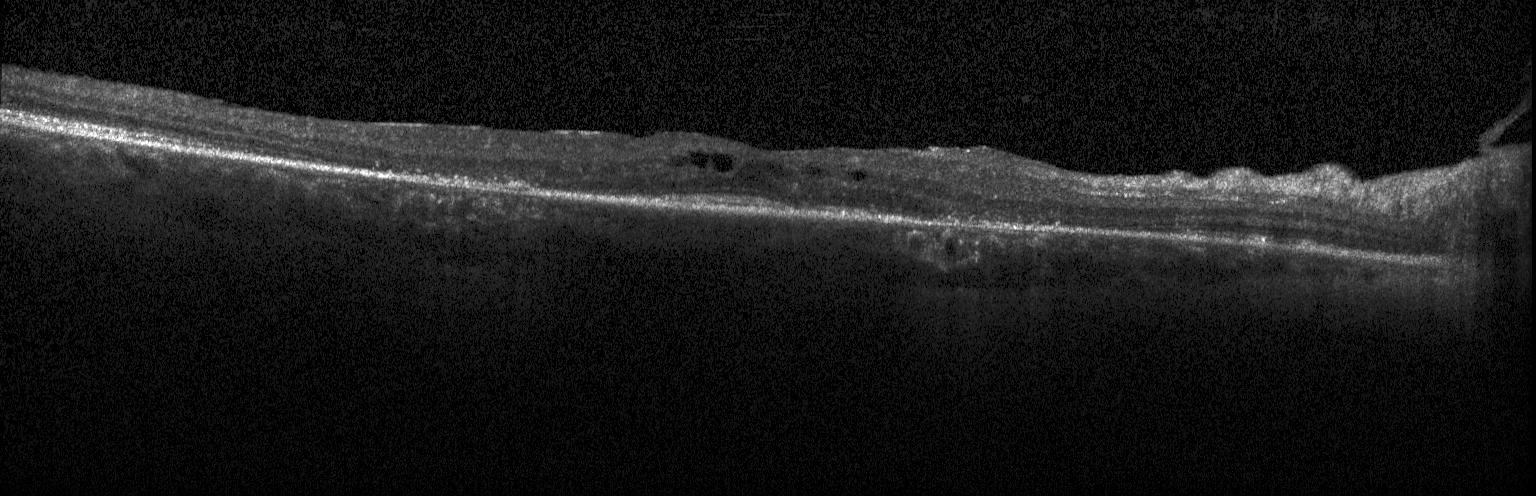

OCT line scan; Heidelberg Spectralis OCT system; fovea-centered — Diagnosis: diabetic macular edema.